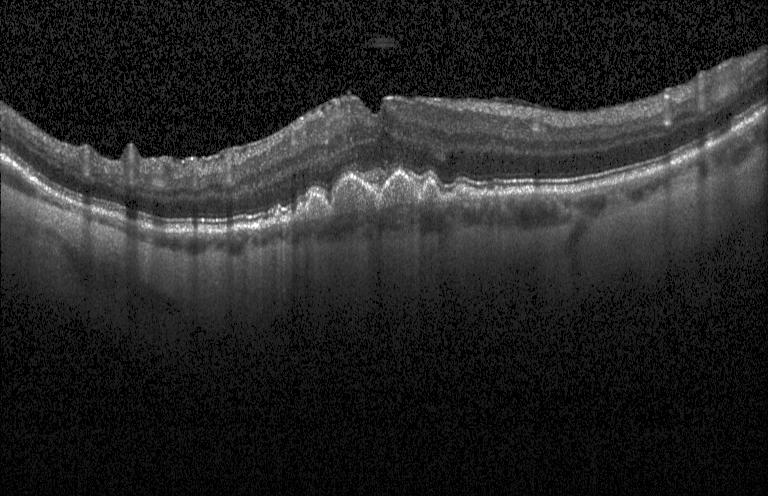
The scan shows drusen.